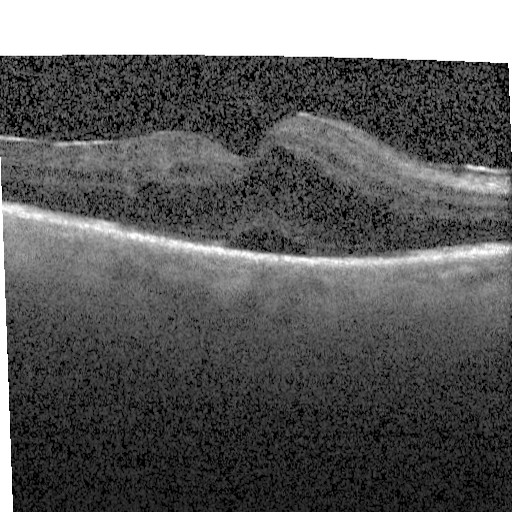
Through the macula, OCT line scan.
This B-scan demonstrates diabetic macular edema (DME).